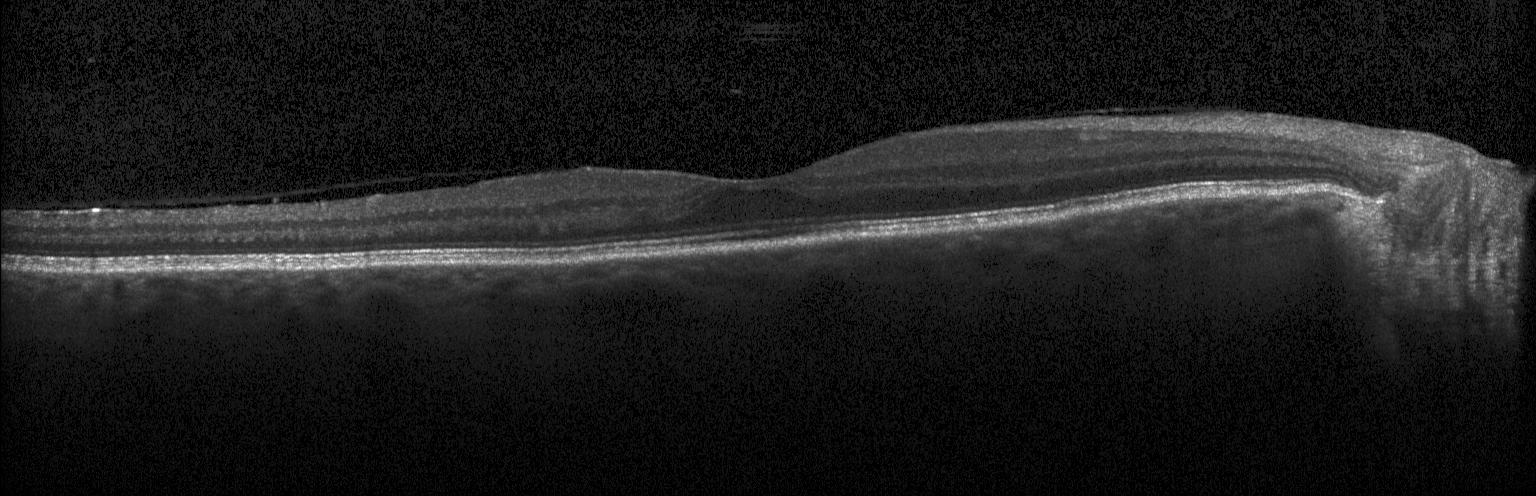

OCT finding: no CNV, no DME, and no drusen.